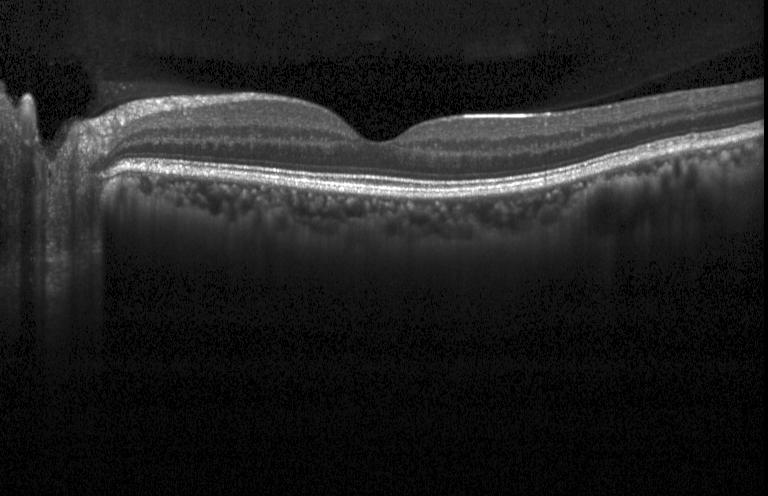

OCT line scan — OCT finding: no CNV, no DME, and no drusen.